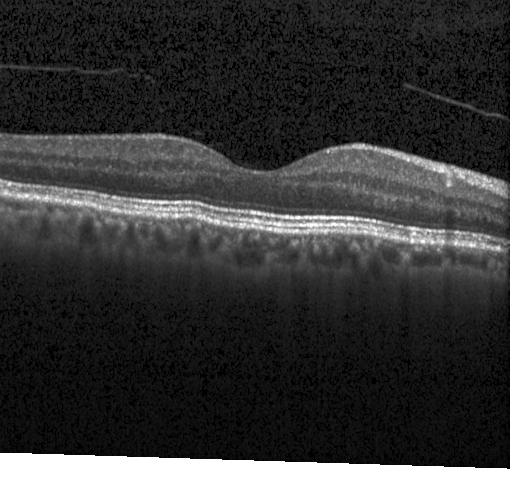 SD-OCT; instrument: Heidelberg Spectralis; OCT B-scan; horizontal scan through the fovea. Impression: no evidence of choroidal neovascularization, diabetic macular edema, or drusen.